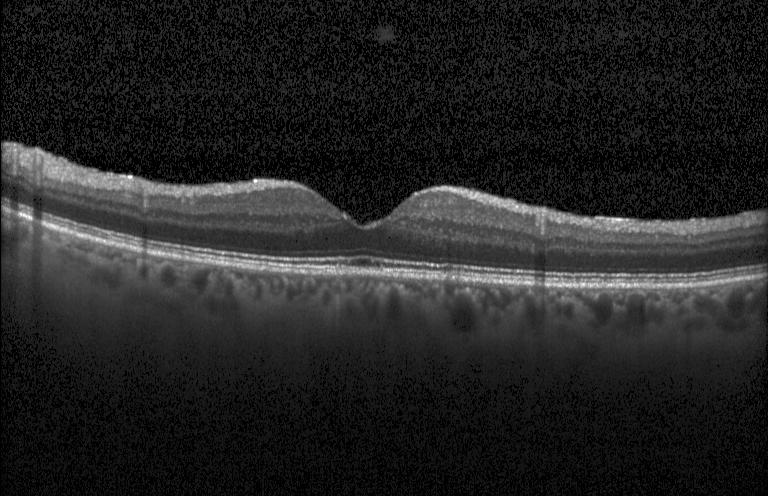

Horizontal scan through the fovea; Heidelberg Spectralis OCT system; OCT line scan. Finding: no choroidal neovascularization, diabetic macular edema, or drusen.